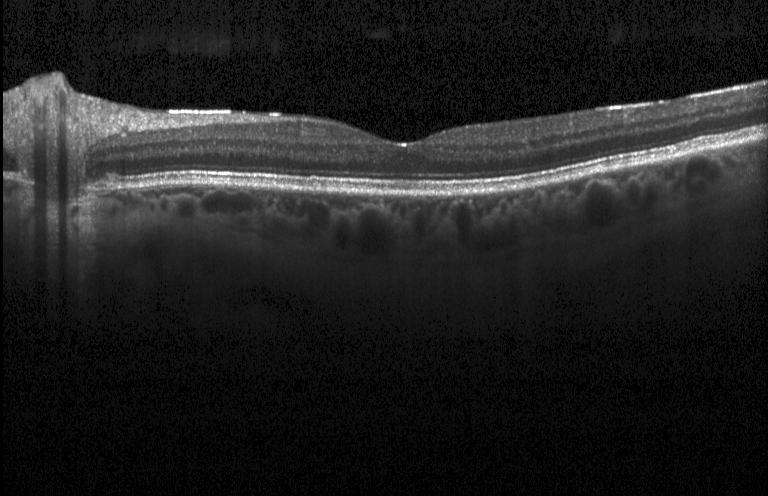
Retinal OCT B-scan; SD-OCT — Assessment: neither choroidal neovascularization, diabetic macular edema, nor drusen.